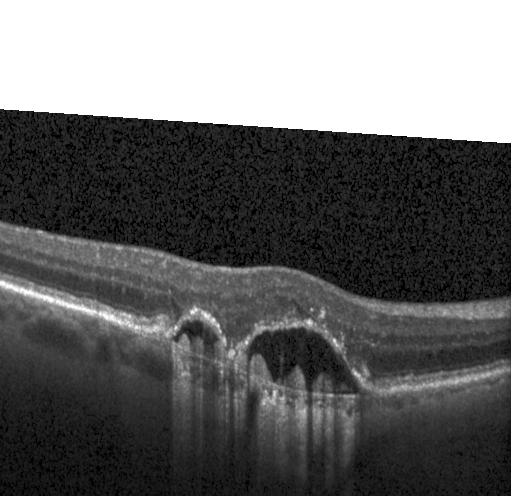

OCT B-scan · Heidelberg Spectralis OCT system.
Finding: choroidal neovascularization.